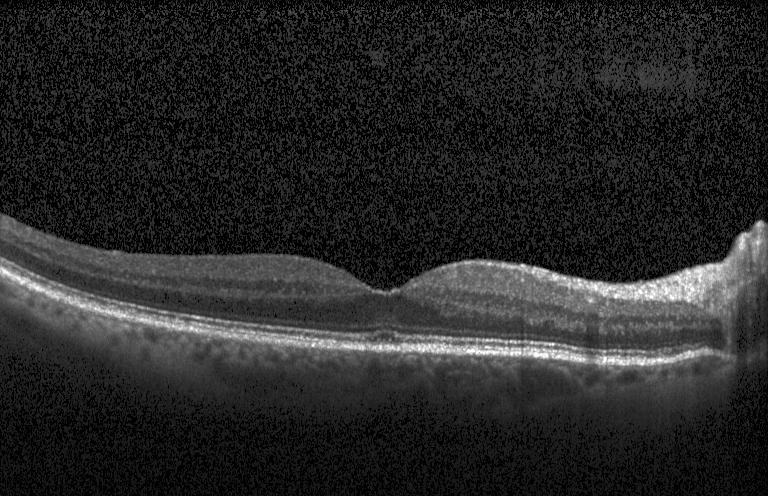
Instrument: Heidelberg Spectralis. Centered on the fovea. Optical coherence tomography scan. Spectral-domain optical coherence tomography — Finding: no evidence of choroidal neovascularization, diabetic macular edema, or drusen.